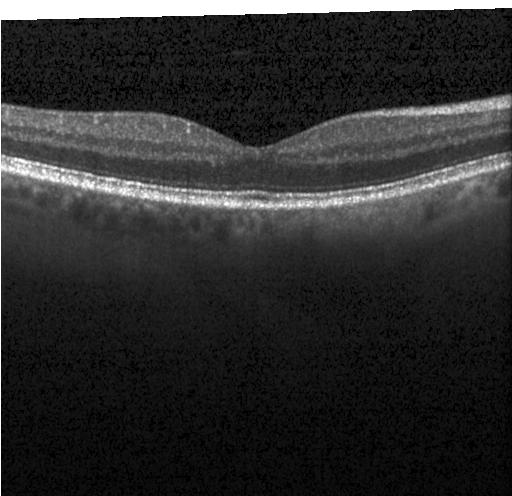
Diagnosis: neither CNV, DME, nor drusen.